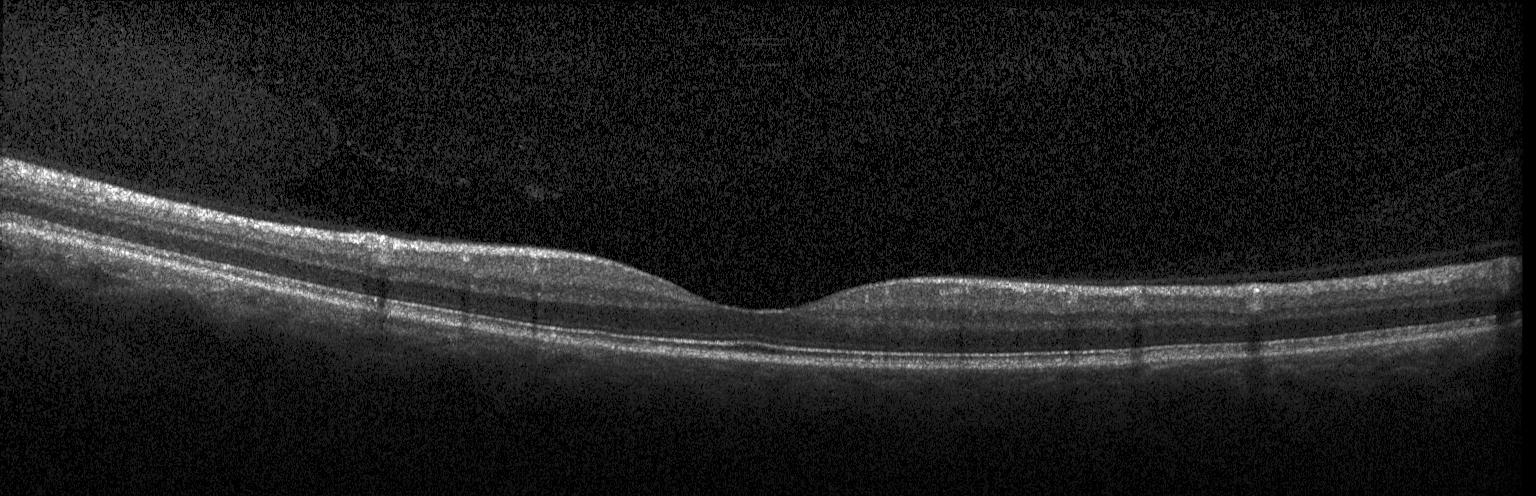 Optical coherence tomography scan
Impression: no evidence of choroidal neovascularization, diabetic macular edema, or drusen.